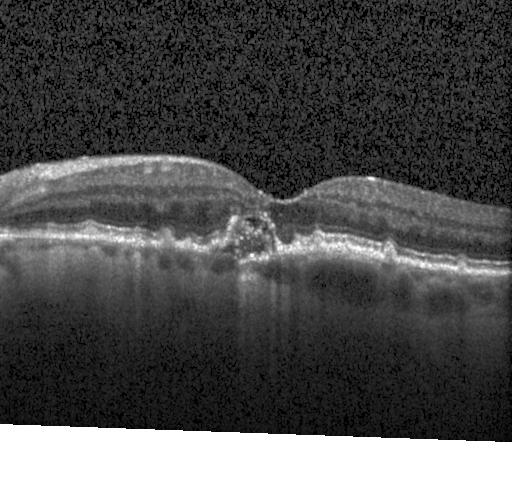

Finding: CNV.